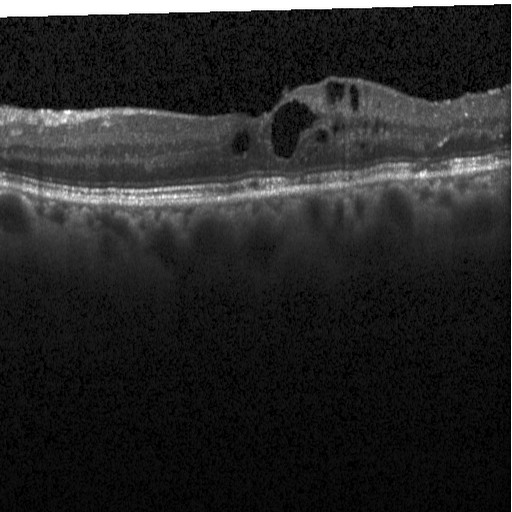

Macular scan · optical coherence tomography B-scan — Finding: DME.